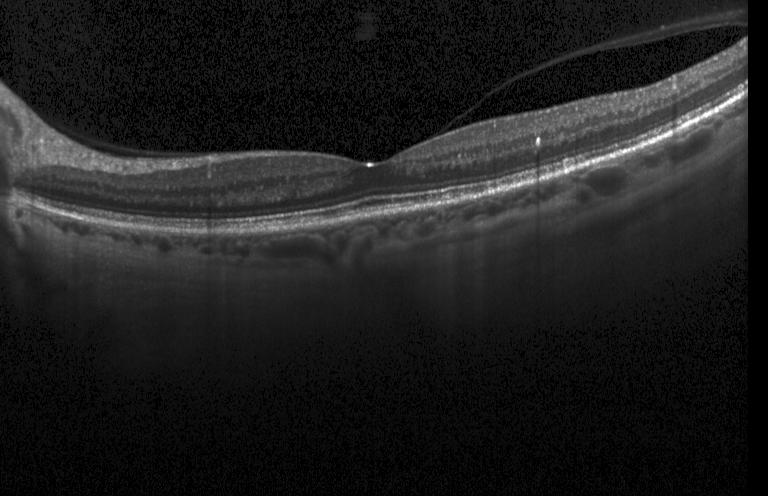
OCT B-scan; spectral-domain optical coherence tomography — Diagnosis: no CNV, DME, or drusen.